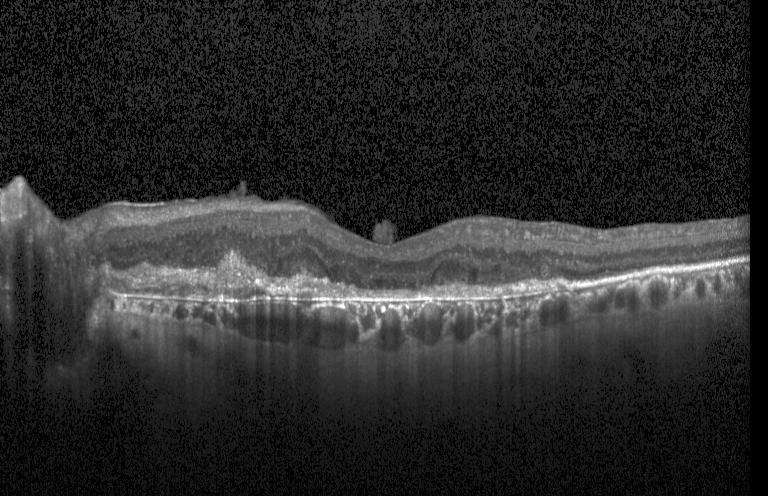 Retinal OCT cross-section — Macular OCT: choroidal neovascularization.